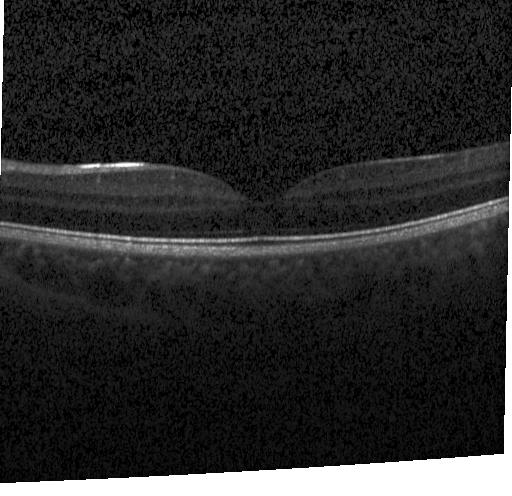 OCT B-scan; Heidelberg Spectralis OCT system — Macular OCT: no choroidal neovascularization, no diabetic macular edema, and no drusen.